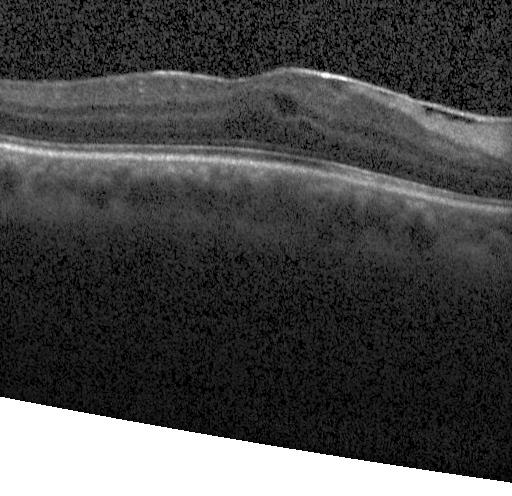 The scan shows diabetic macular edema.